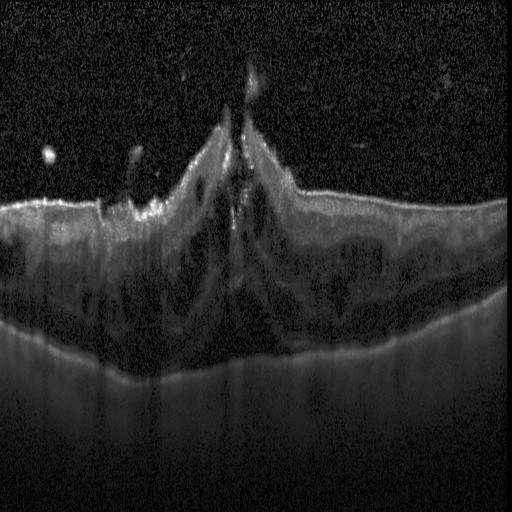 OCT line scan; spectral-domain optical coherence tomography; Heidelberg Spectralis. OCT finding: diabetic macular edema.